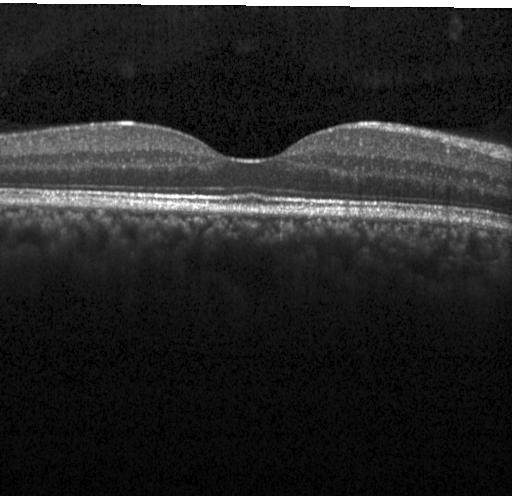
This B-scan demonstrates neither choroidal neovascularization, diabetic macular edema, nor drusen.